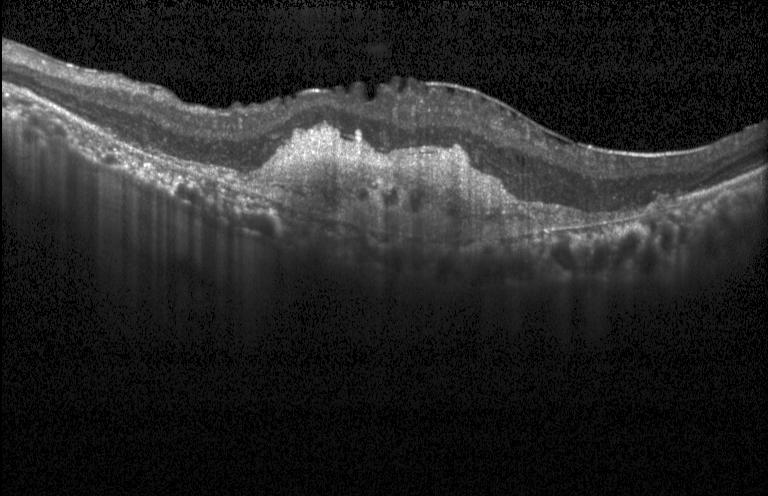

OCT line scan — Macular OCT: a choroidal neovascular membrane.